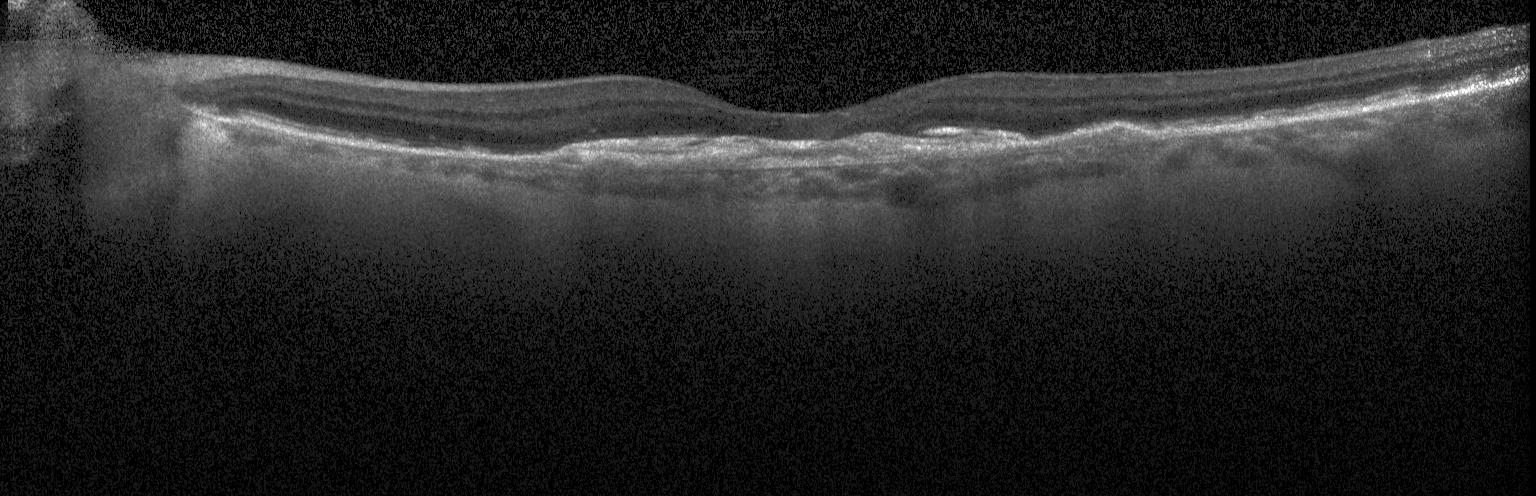
Through the macula. Instrument: Heidelberg Spectralis. Optical coherence tomography B-scan
The scan shows choroidal neovascularization.